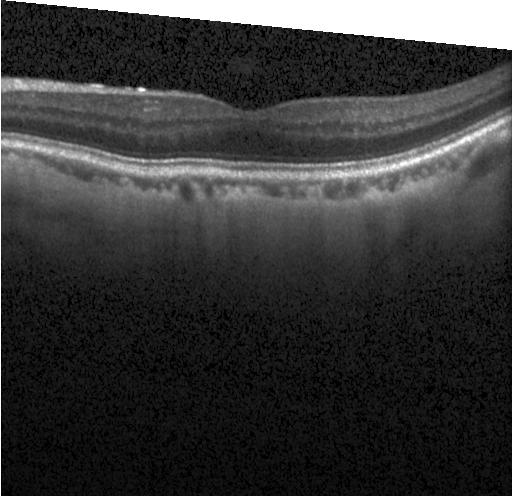

SD-OCT, optical coherence tomography scan, horizontal scan through the fovea, acquired on a Heidelberg Spectralis — Finding: no choroidal neovascularization, no diabetic macular edema, and no drusen.